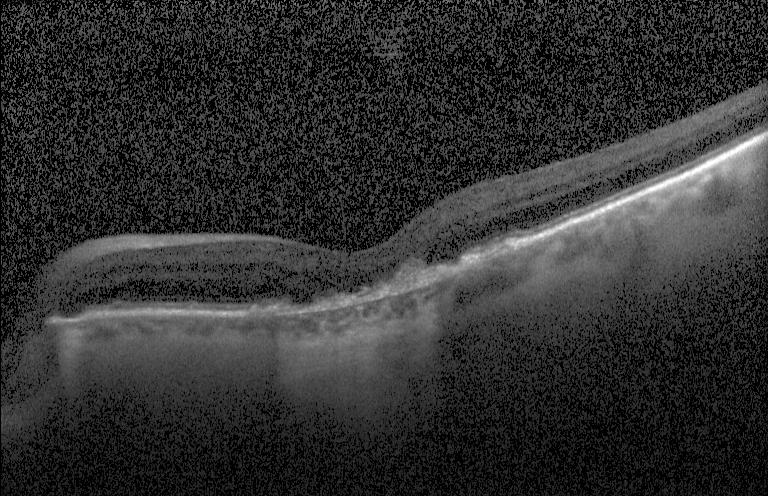
Diagnosis: a choroidal neovascular membrane.